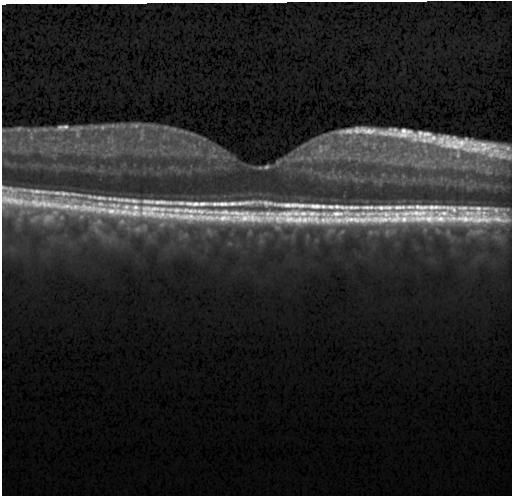 Finding: no evidence of choroidal neovascularization, diabetic macular edema, or drusen.